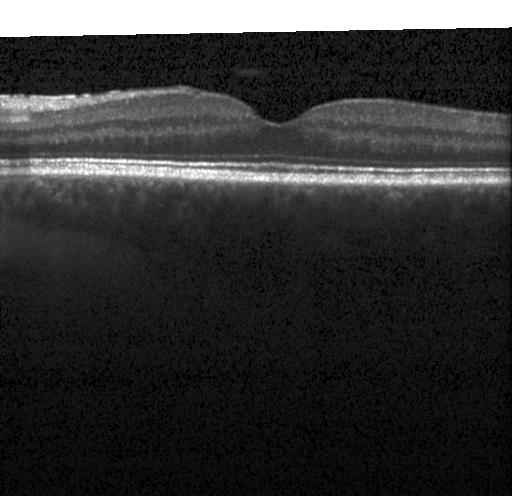 OCT line scan.
Finding: no evidence of CNV, DME, or drusen.